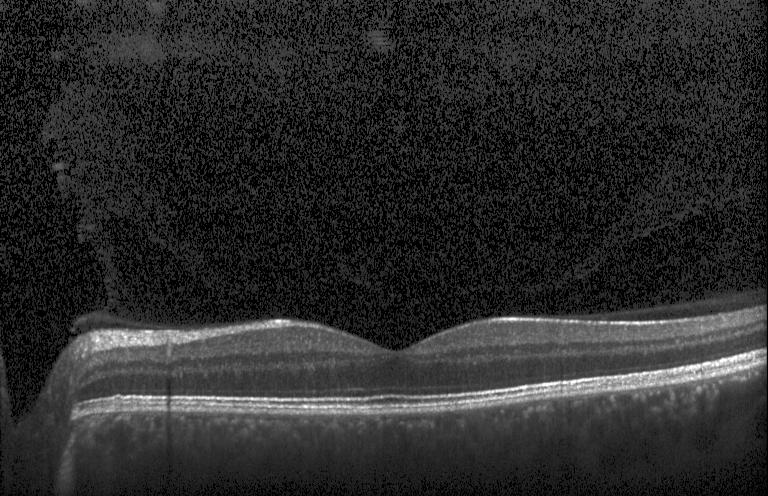

Optical coherence tomography scan; Heidelberg Spectralis; spectral-domain OCT. Finding: neither CNV, DME, nor drusen.